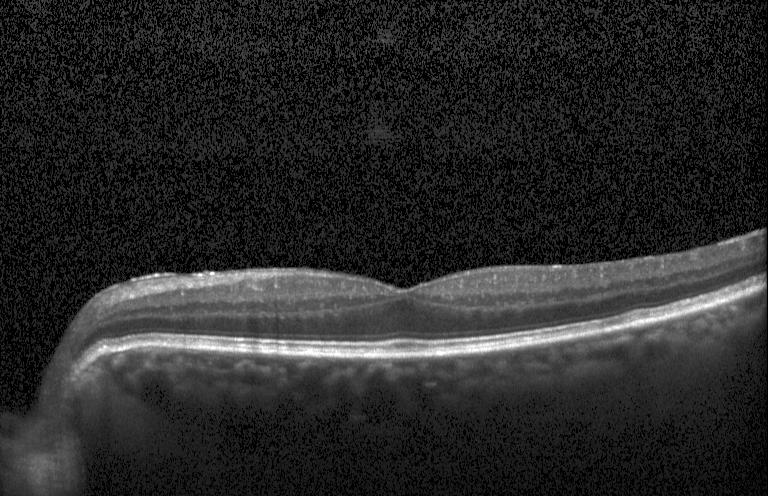
Diagnosis: neither CNV, DME, nor drusen.